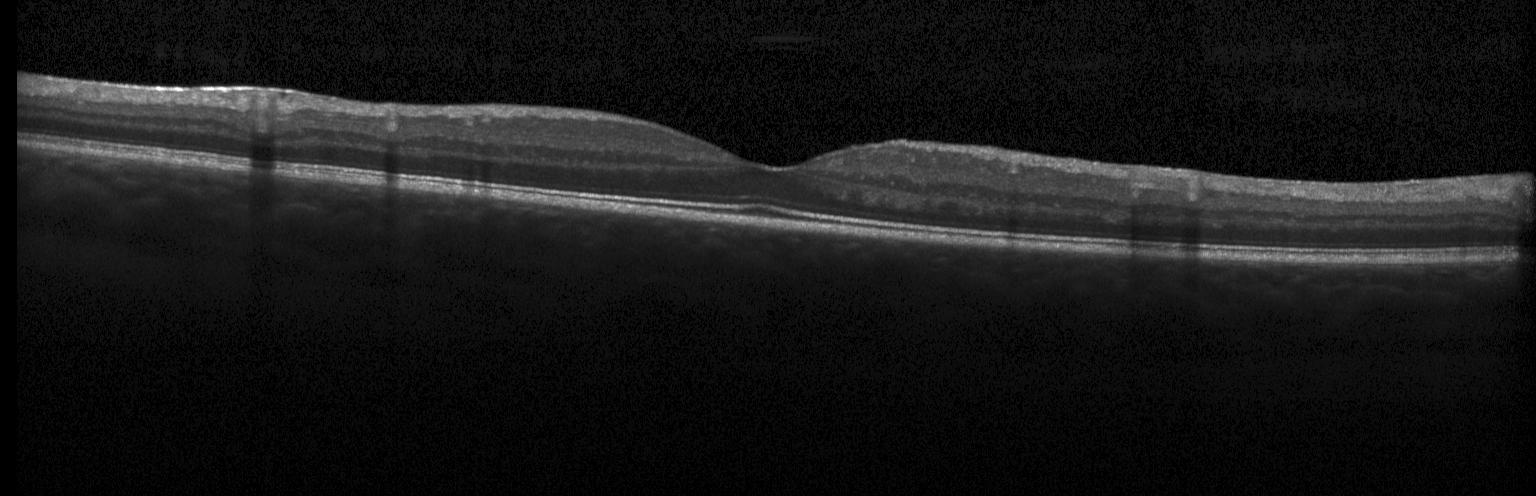 Instrument: Heidelberg Spectralis. Through the macula. Spectral-domain OCT. Retinal OCT cross-section — Impression: neither choroidal neovascularization, diabetic macular edema, nor drusen.